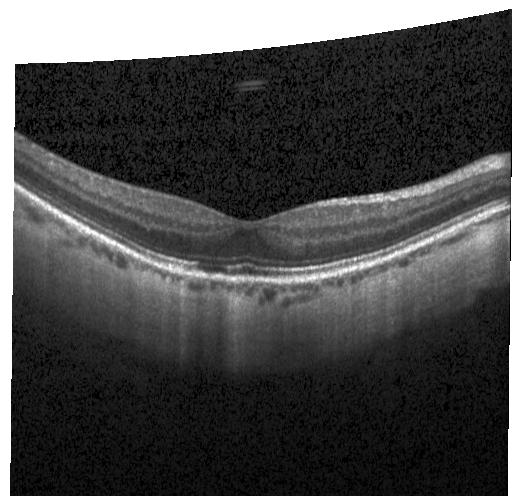
OCT line scan · through the macula · Heidelberg Spectralis — Macular OCT: no choroidal neovascularization, diabetic macular edema, or drusen.